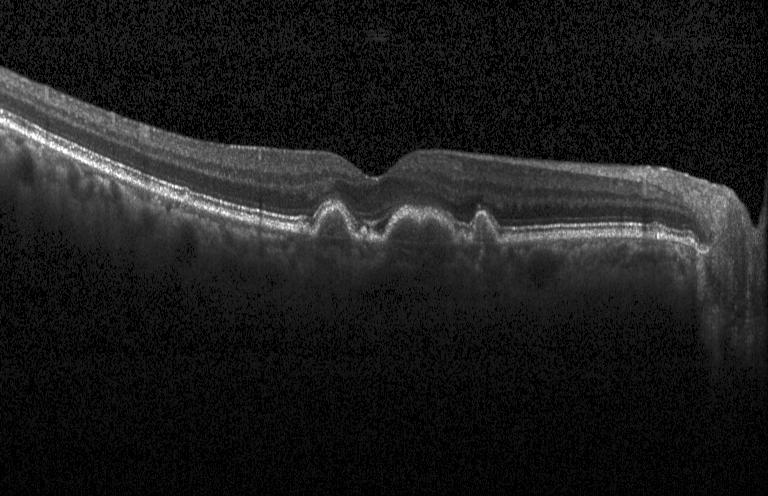
Dx: drusen.